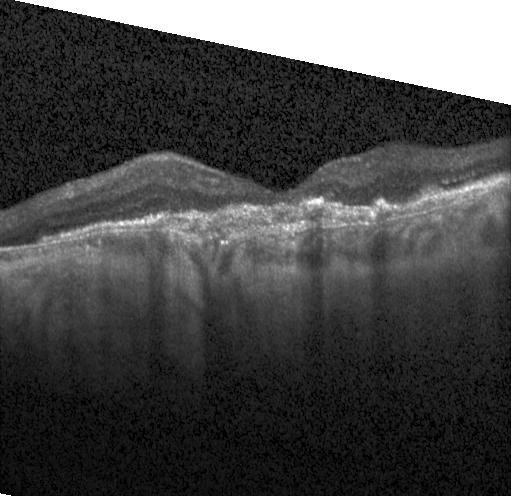

Spectral-domain optical coherence tomography, Heidelberg Spectralis OCT system, optical coherence tomography B-scan, macular scan. A choroidal neovascular membrane.